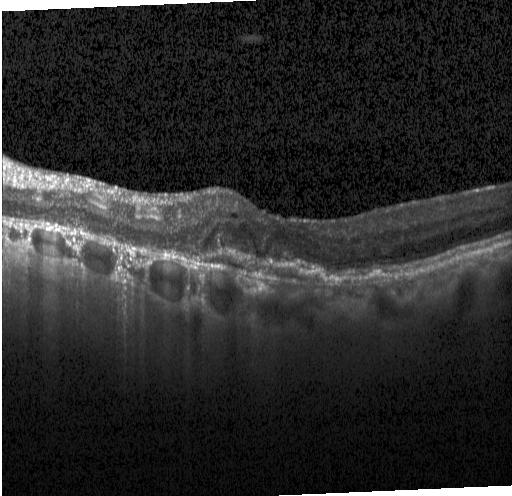
Impression: choroidal neovascularization.